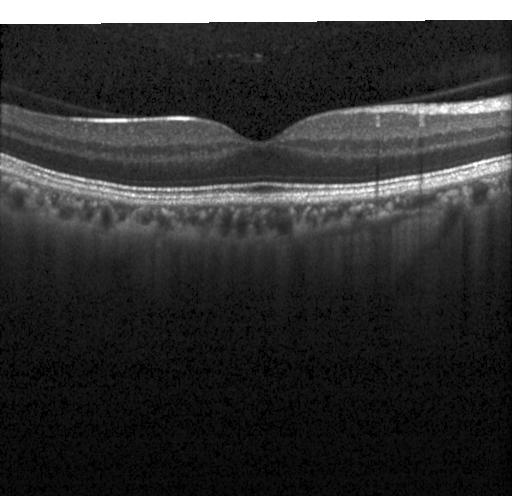 SD-OCT · OCT B-scan
No evidence of choroidal neovascularization, diabetic macular edema, or drusen.